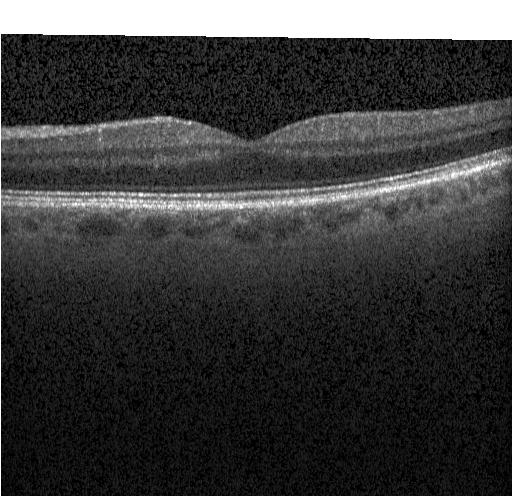 Macular OCT: no evidence of choroidal neovascularization, diabetic macular edema, or drusen.